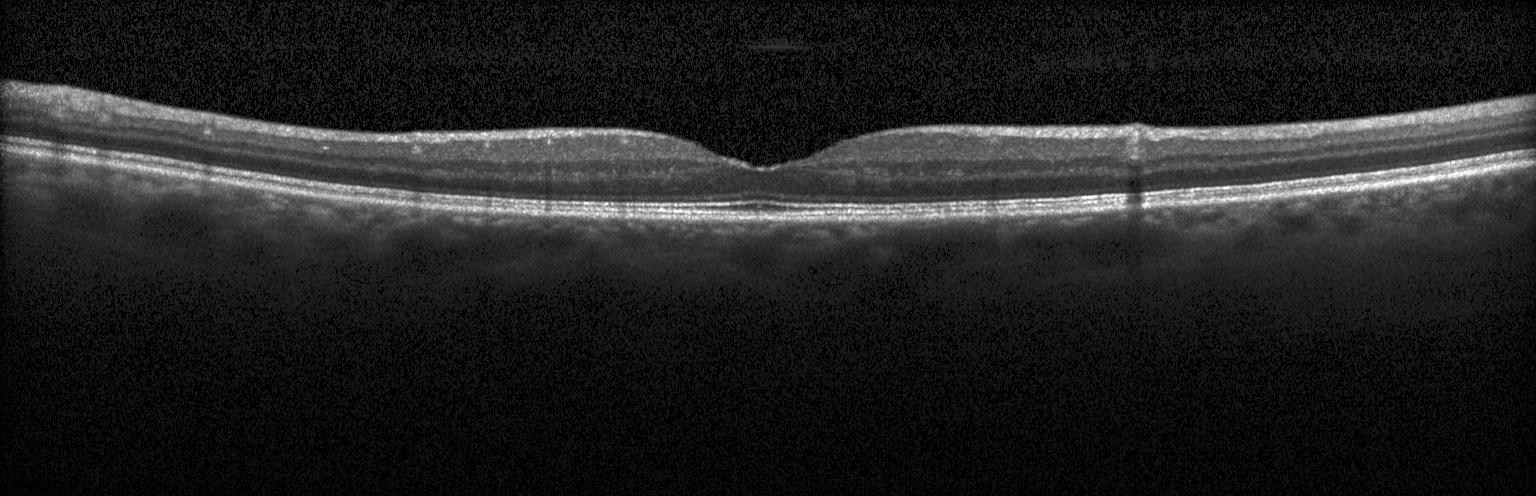

Optical coherence tomography scan, instrument: Heidelberg Spectralis — No choroidal neovascularization, diabetic macular edema, or drusen.